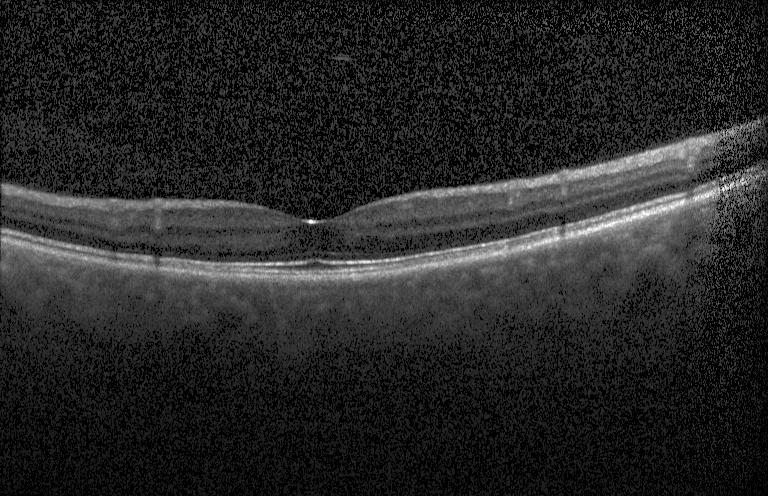
Acquired on a Heidelberg Spectralis. Optical coherence tomography B-scan. Macular scan.
Assessment: no choroidal neovascularization, diabetic macular edema, or drusen.